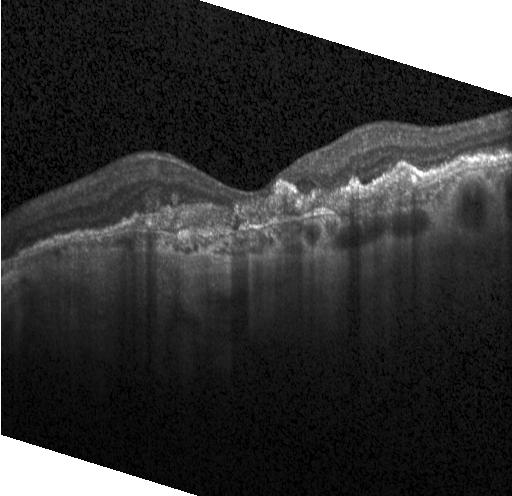
Instrument: Heidelberg Spectralis; optical coherence tomography scan
Macular OCT: a choroidal neovascular membrane.